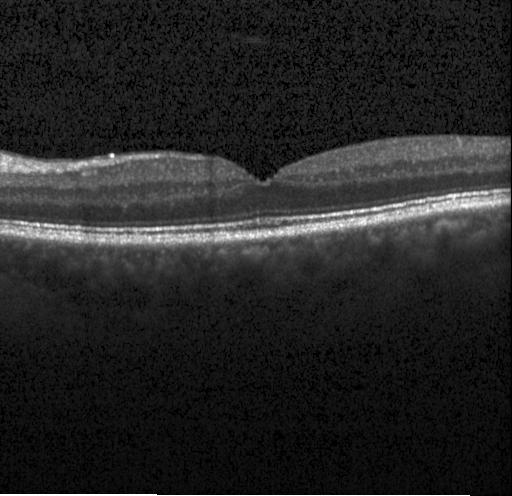 Centered on the fovea. Optical coherence tomography scan. The scan shows neither CNV, DME, nor drusen.